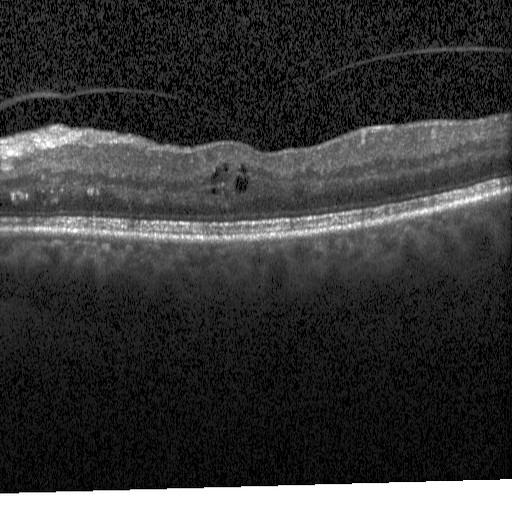
Spectral-domain OCT B-scan: DME.